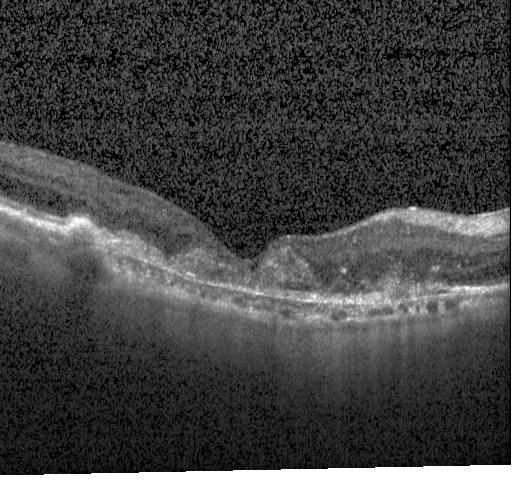 OCT B-scan · macular scan · spectral-domain optical coherence tomography
Finding: a choroidal neovascular membrane.